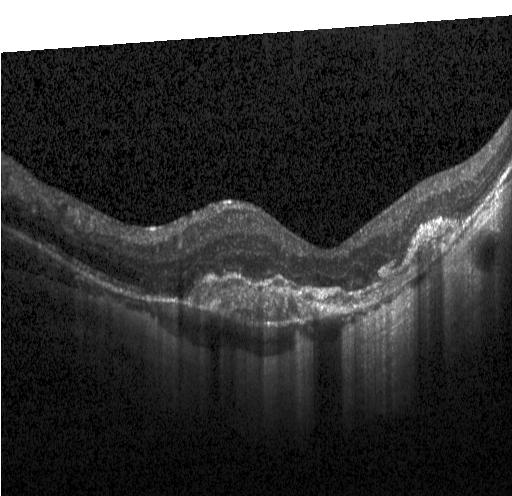

The scan shows CNV.